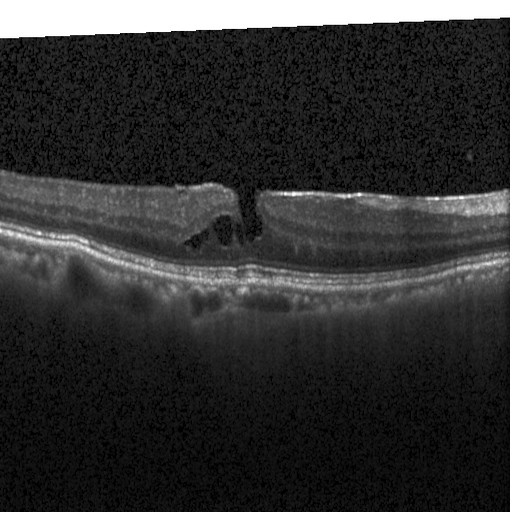

Dx: diabetic macular edema.